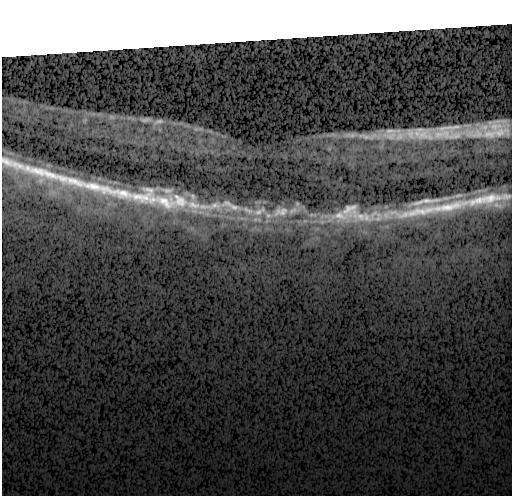
Spectral-domain optical coherence tomography; acquired on a Heidelberg Spectralis; fovea-centered; retinal OCT cross-section
Finding: CNV.